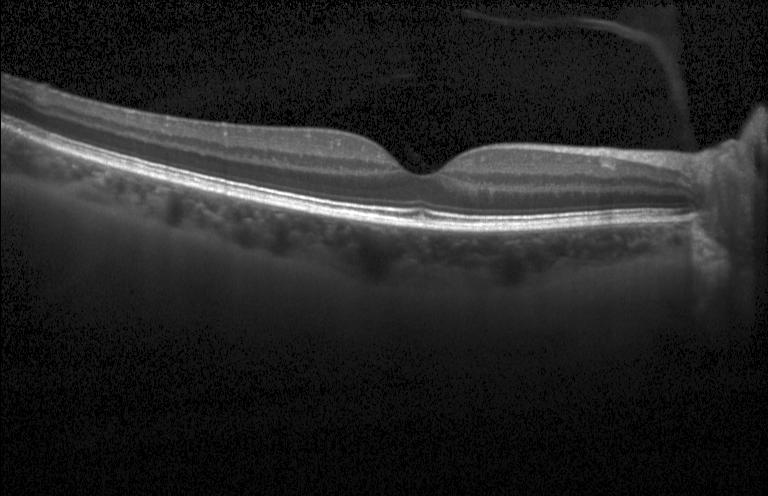 Retinal OCT cross-section.
Macular OCT: neither choroidal neovascularization, diabetic macular edema, nor drusen.